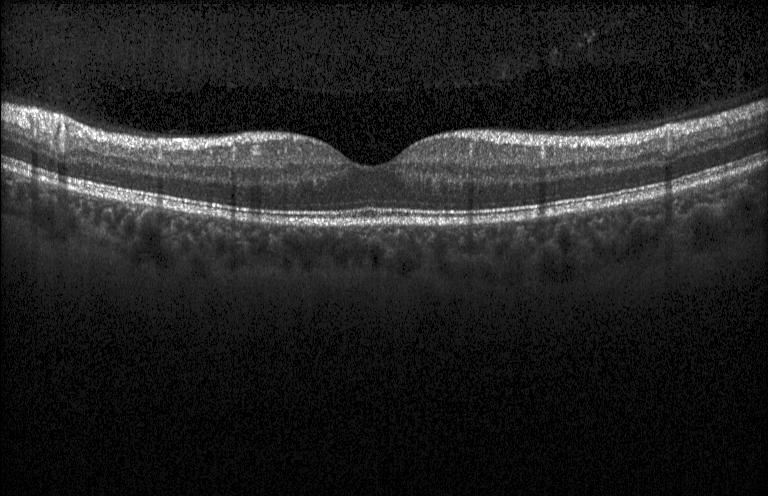

Neither CNV, DME, nor drusen.